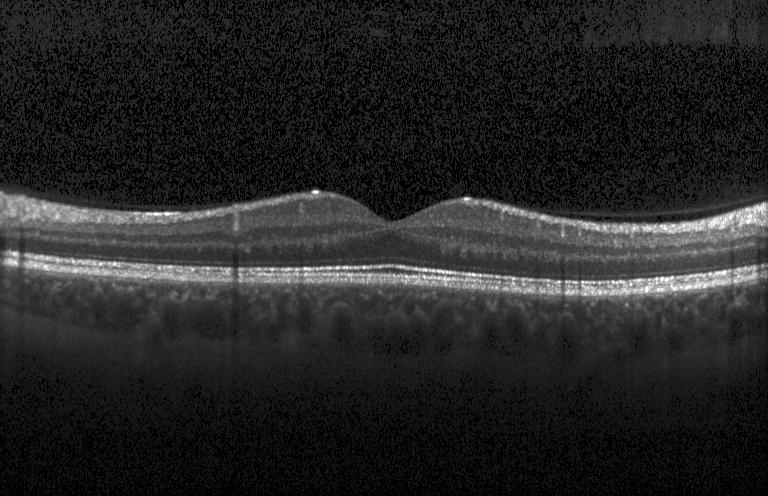

Retinal OCT B-scan. Impression: neither choroidal neovascularization, diabetic macular edema, nor drusen.